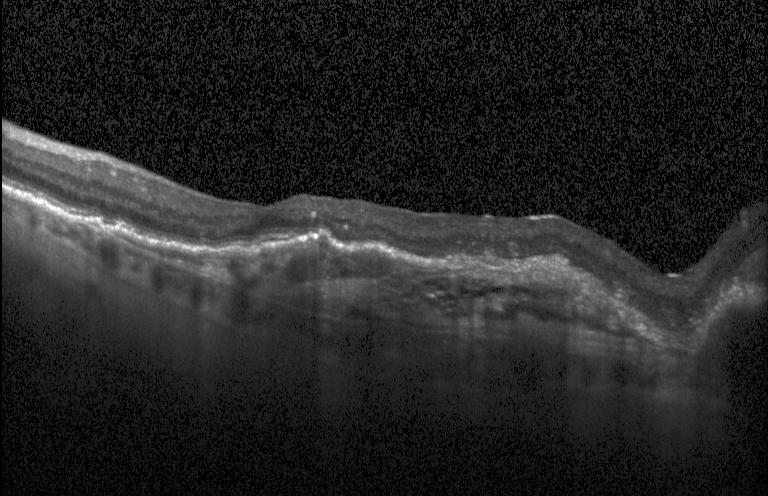 Heidelberg Spectralis, retinal OCT cross-section, spectral-domain OCT. OCT finding: CNV.